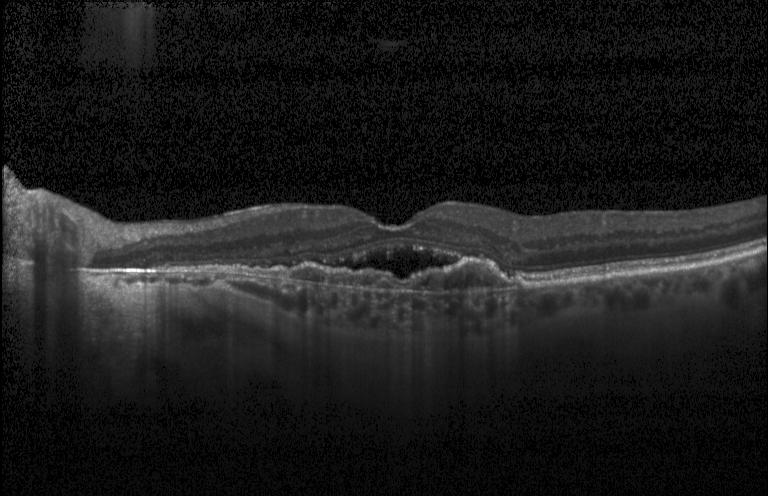 Macular OCT: a choroidal neovascular membrane.